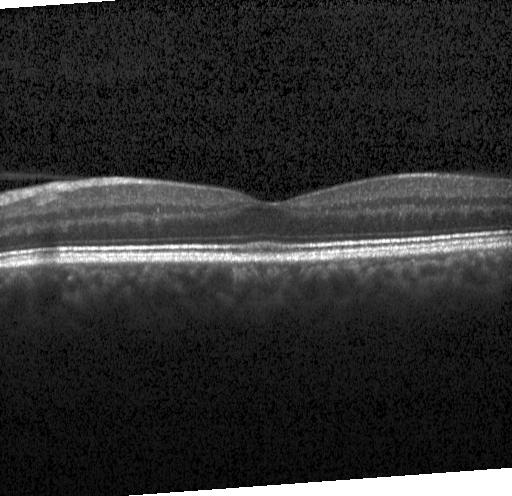 Optical coherence tomography B-scan
Finding: no CNV, DME, or drusen.